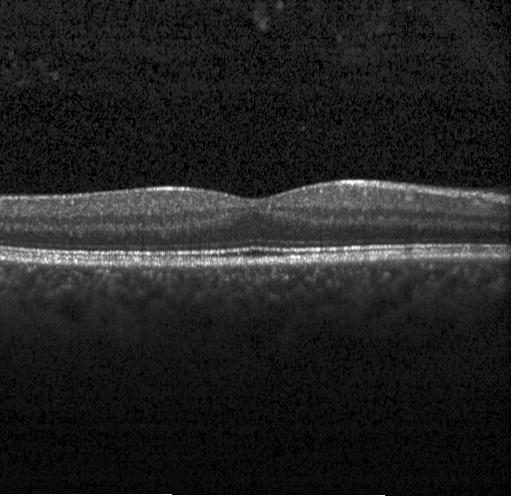 Acquired on a Heidelberg Spectralis, retinal OCT B-scan
Dx: neither choroidal neovascularization, diabetic macular edema, nor drusen.